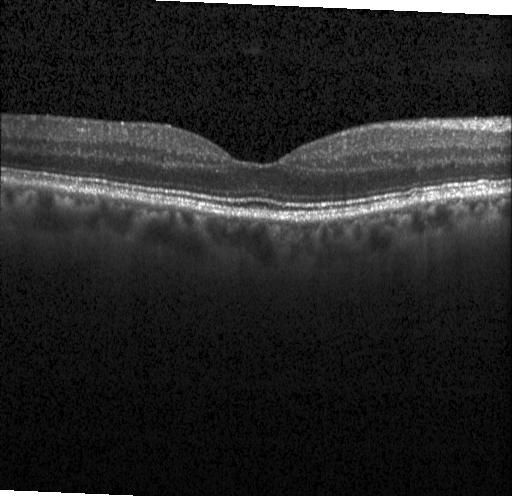 Optical coherence tomography B-scan.
Assessment: neither choroidal neovascularization, diabetic macular edema, nor drusen.